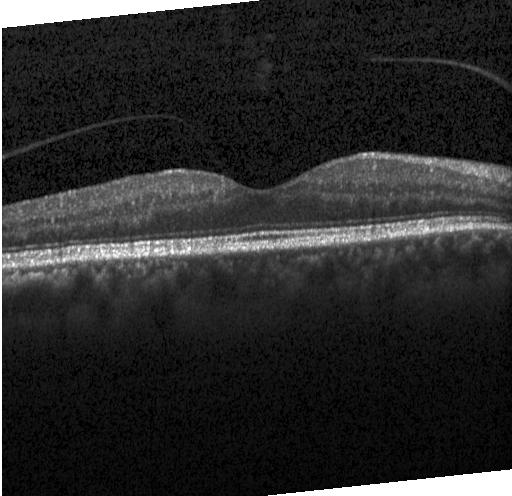

Optical coherence tomography B-scan, Heidelberg Spectralis OCT system. OCT finding: no CNV, DME, or drusen.